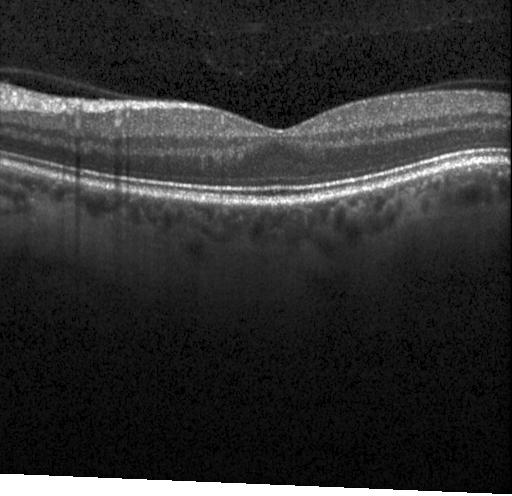
Optical coherence tomography B-scan, Heidelberg Spectralis OCT system — Diagnosis: no CNV, DME, or drusen.